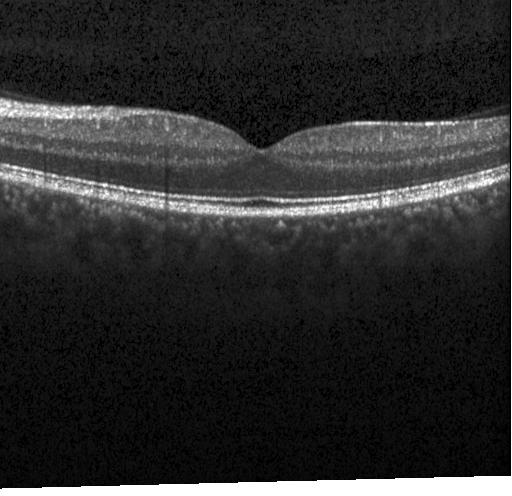
Optical coherence tomography scan.
Finding: no CNV, DME, or drusen.